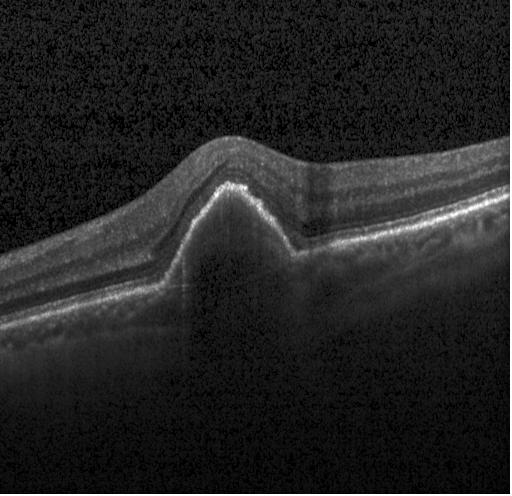

SD-OCT · through the macula · OCT B-scan
Diagnosis: a choroidal neovascular membrane.